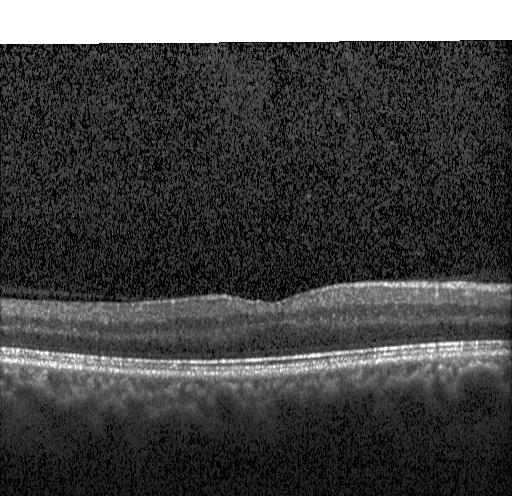
Instrument: Heidelberg Spectralis, spectral-domain OCT, OCT line scan — Finding: no choroidal neovascularization, no diabetic macular edema, and no drusen.